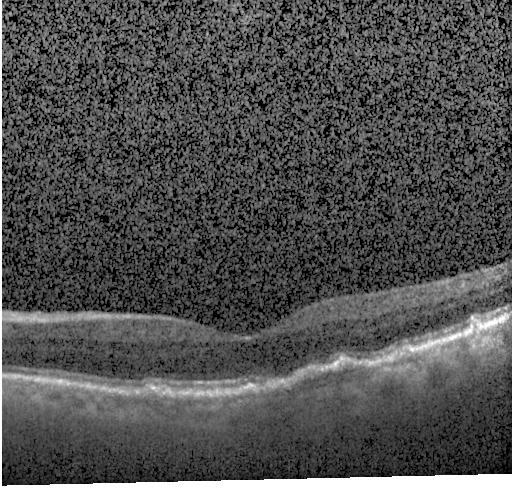

Heidelberg Spectralis · retinal OCT B-scan · fovea-centered.
Impression: choroidal neovascularization.